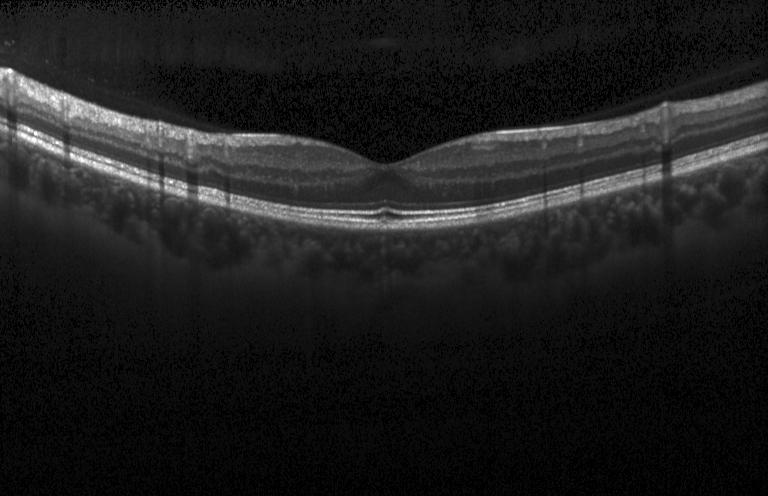
Heidelberg Spectralis, retinal OCT cross-section, fovea-centered, SD-OCT.
Finding: no CNV, no DME, and no drusen.